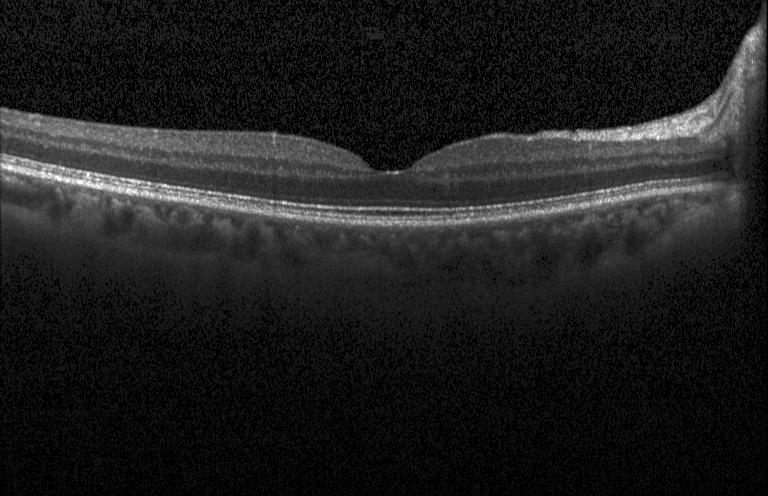

Diagnosis: no evidence of CNV, DME, or drusen.